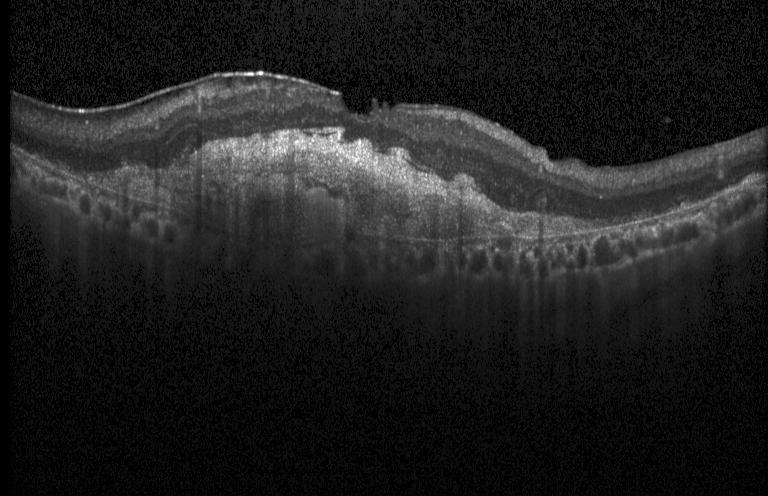 Retinal OCT B-scan. Diagnosis: choroidal neovascularization (CNV).